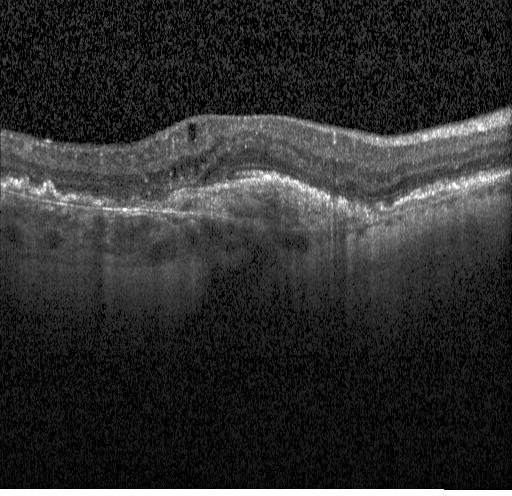
Macular OCT: CNV.